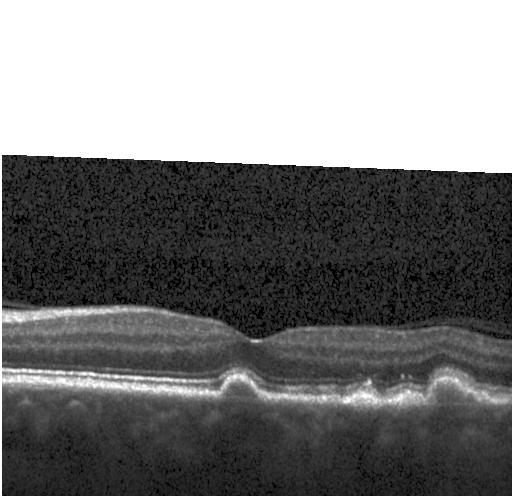

Diagnosis: multiple drusen.